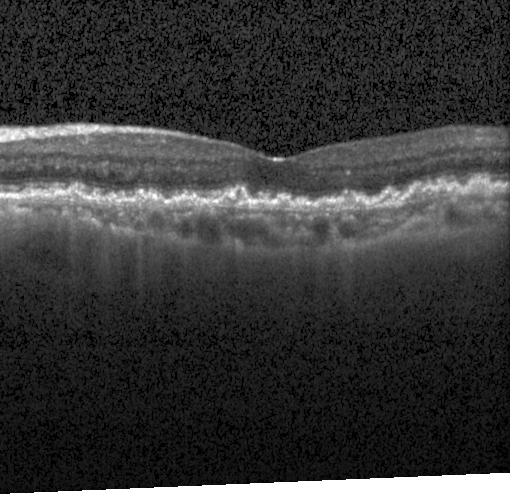
Finding: multiple drusen.